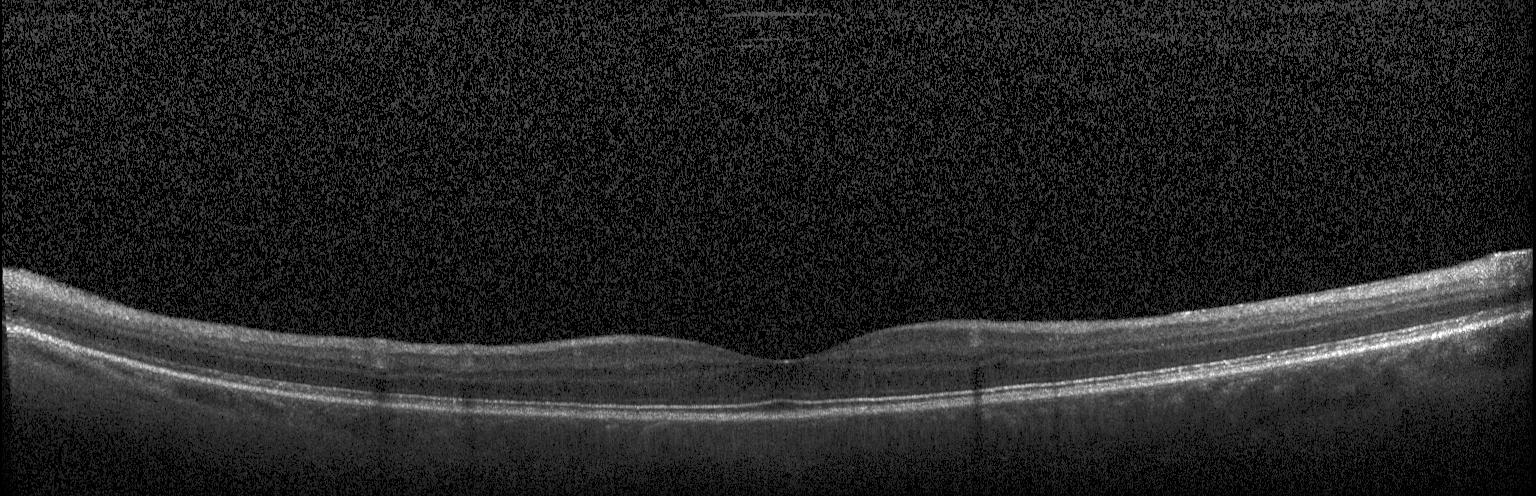 Through the macula, spectral-domain OCT, instrument: Heidelberg Spectralis, retinal OCT B-scan — Dx: no CNV, no DME, and no drusen.